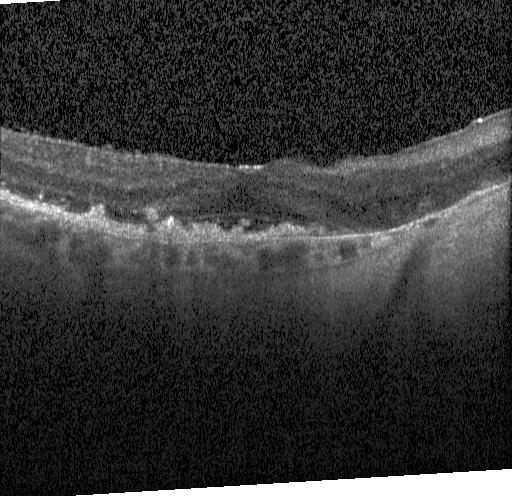
Retinal OCT cross-section. Instrument: Heidelberg Spectralis. SD-OCT. Fovea-centered — Macular OCT: a choroidal neovascular membrane.